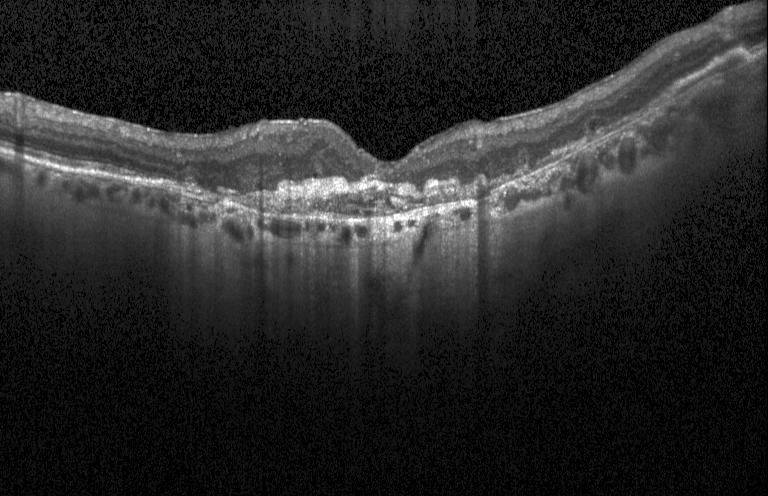

The scan shows a choroidal neovascular membrane.